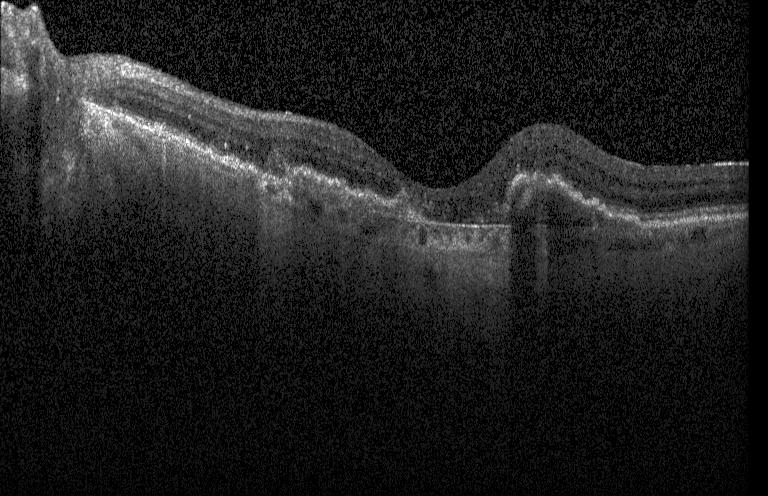
Macular scan · Heidelberg Spectralis OCT system · OCT line scan · spectral-domain optical coherence tomography — This B-scan demonstrates a choroidal neovascular membrane.